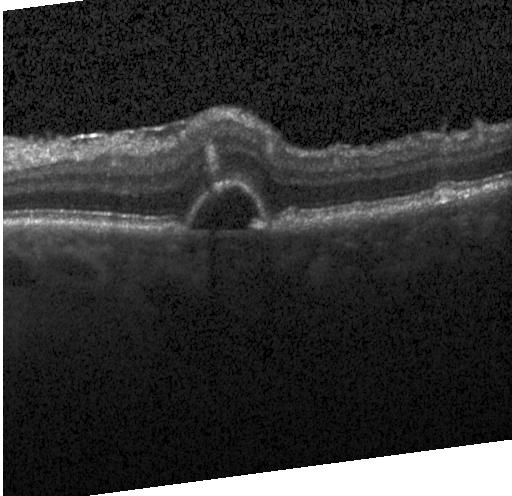 Instrument: Heidelberg Spectralis, retinal OCT B-scan, centered on the fovea, spectral-domain optical coherence tomography
Dx: a choroidal neovascular membrane.